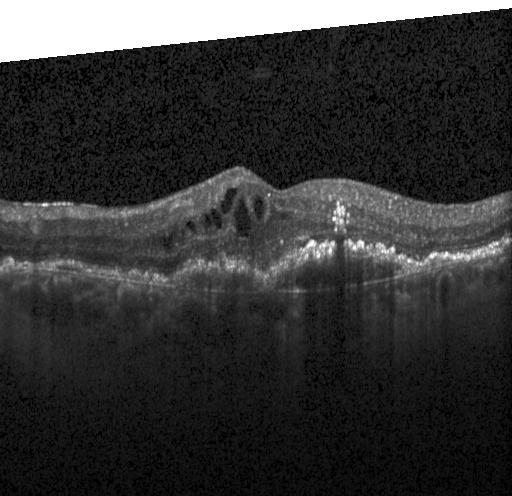 Macular OCT demonstrating a choroidal neovascular membrane.